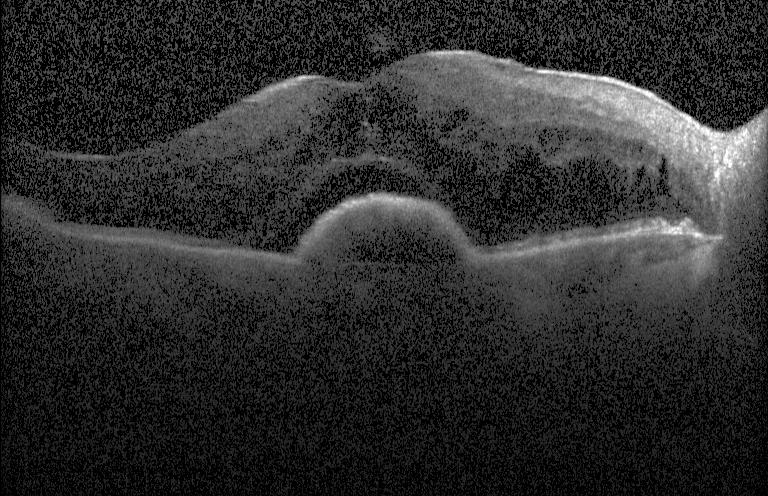
Macular OCT: a choroidal neovascular membrane.